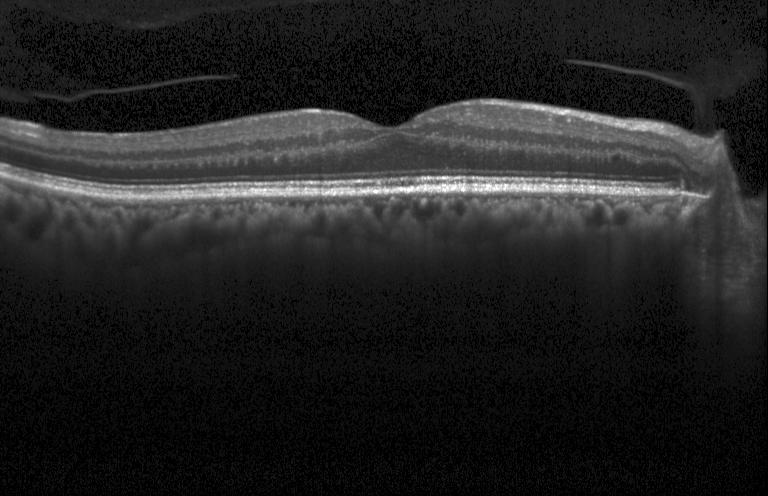

Through the macula · retinal OCT B-scan · acquired on a Heidelberg Spectralis
This B-scan demonstrates neither choroidal neovascularization, diabetic macular edema, nor drusen.